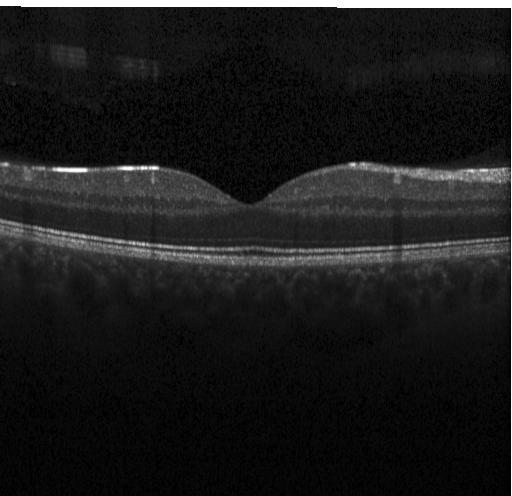 OCT finding: neither choroidal neovascularization, diabetic macular edema, nor drusen.